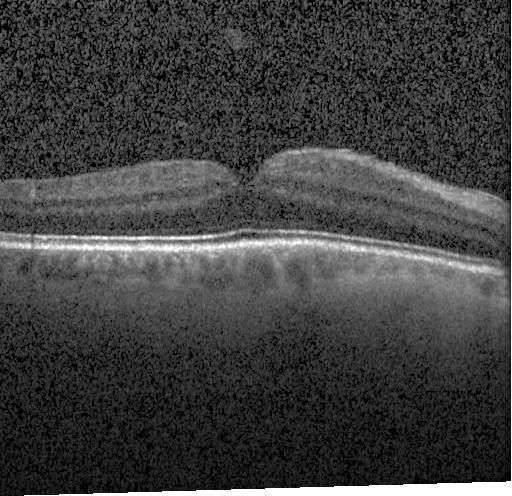
The scan shows no choroidal neovascularization, no diabetic macular edema, and no drusen.